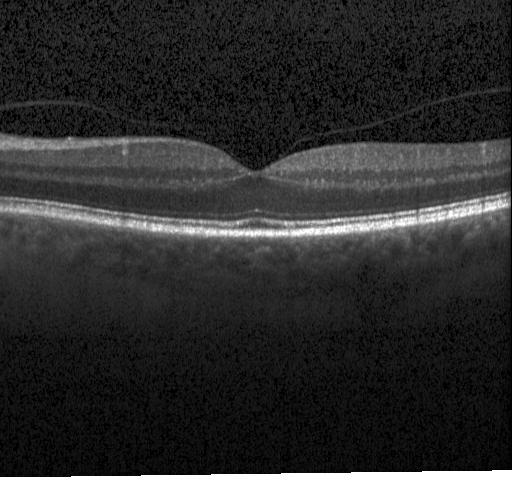

This B-scan demonstrates no evidence of CNV, DME, or drusen.